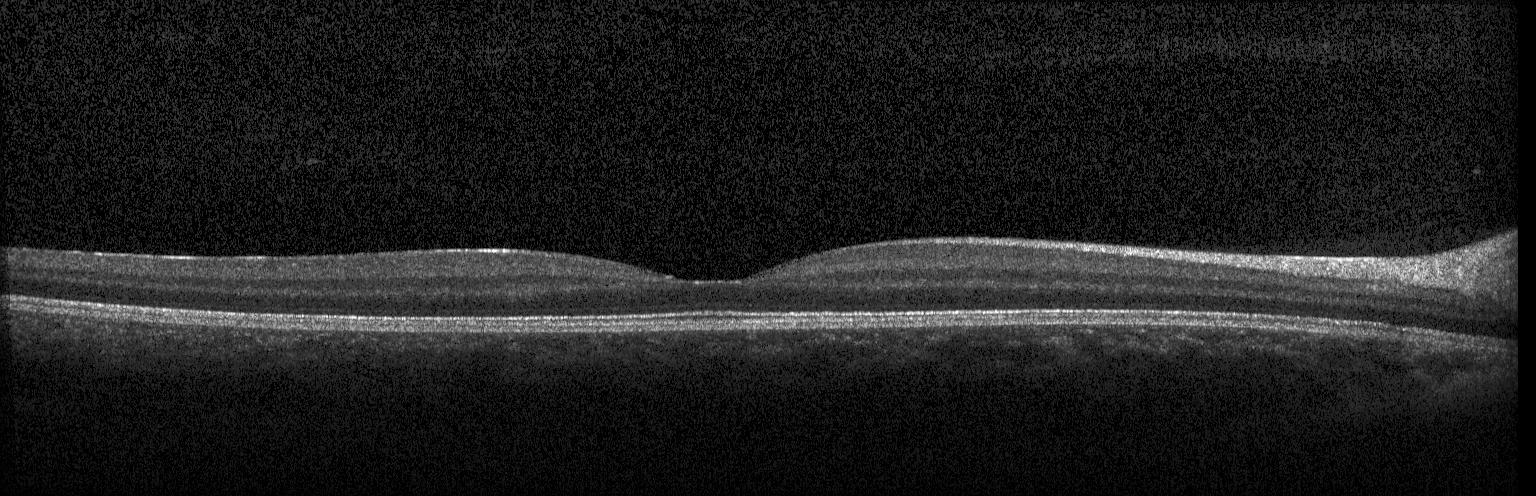 No choroidal neovascularization, no diabetic macular edema, and no drusen.